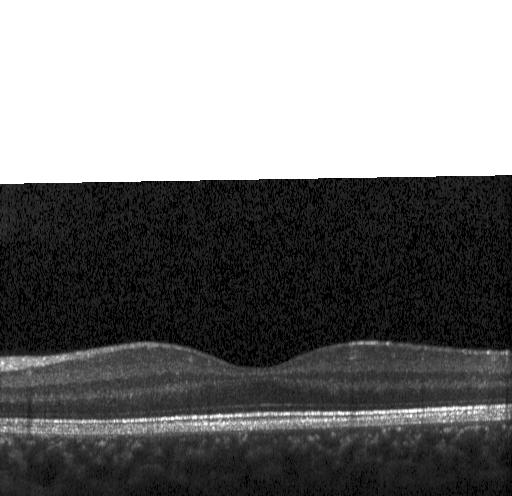

Impression: neither choroidal neovascularization, diabetic macular edema, nor drusen.